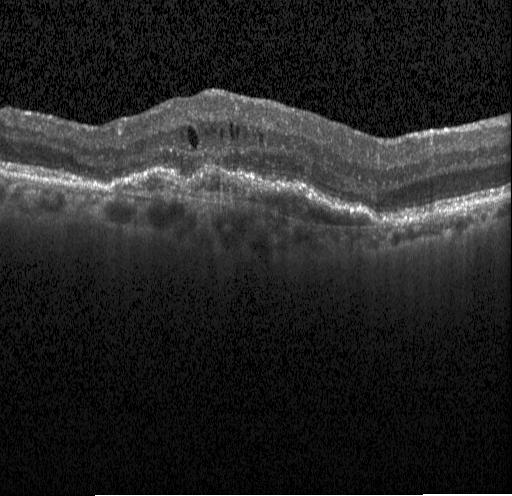
SD-OCT. OCT line scan. Heidelberg Spectralis OCT system
Diagnosis: choroidal neovascularization (CNV).